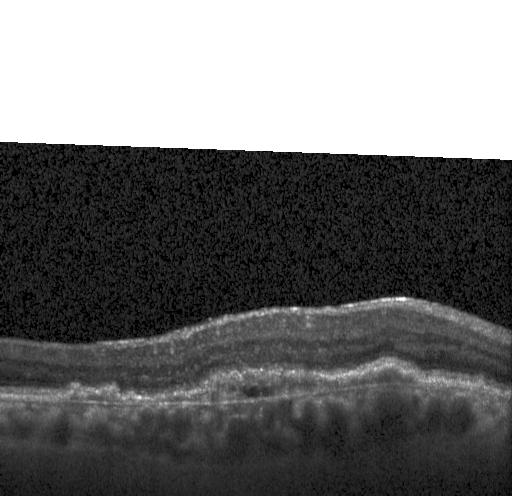
Acquired on a Heidelberg Spectralis. OCT line scan — Diagnosis: a choroidal neovascular membrane.